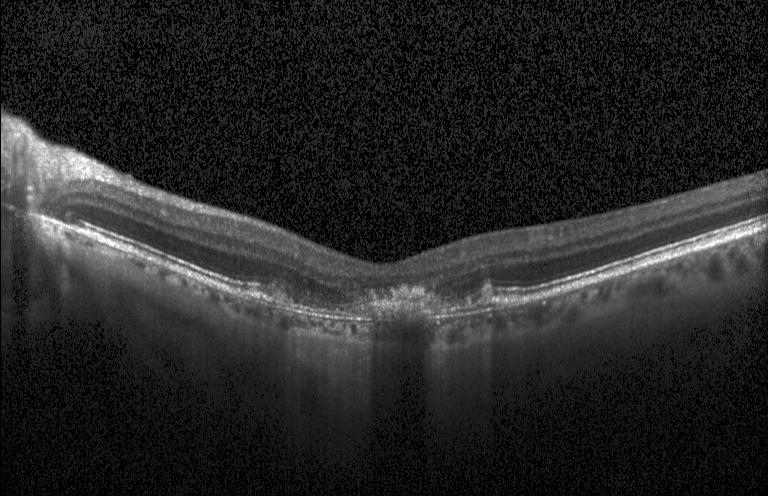

Retinal OCT B-scan
OCT finding: choroidal neovascularization (CNV).